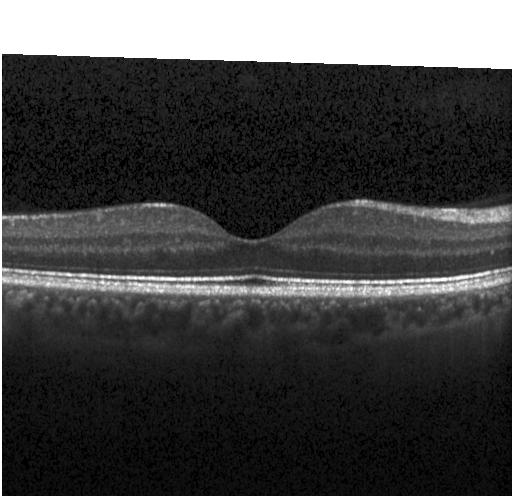

OCT finding: neither CNV, DME, nor drusen.